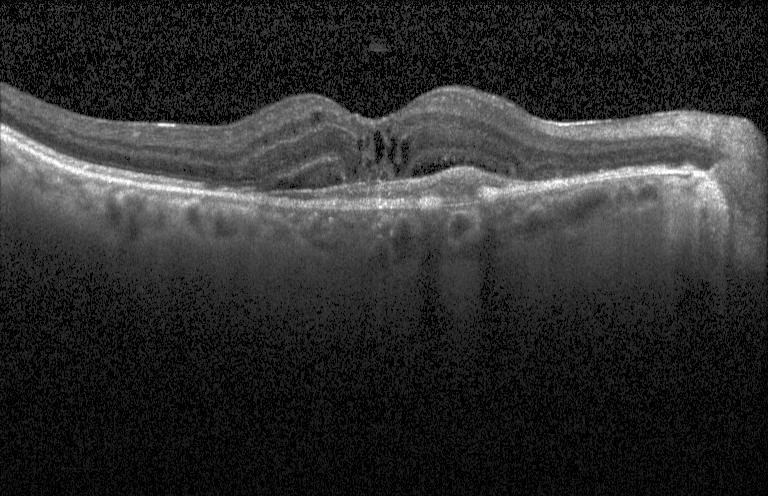
Impression: a choroidal neovascular membrane.